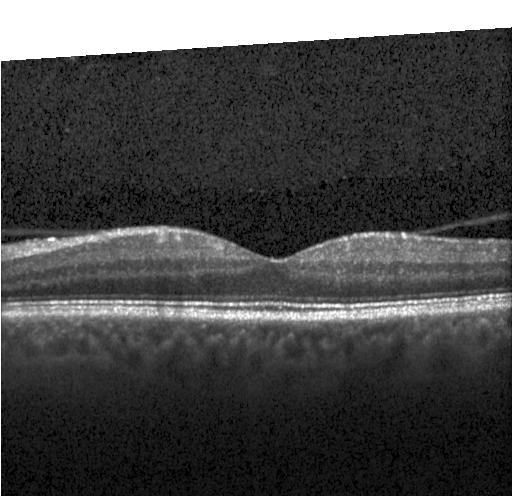

Diagnosis: no evidence of choroidal neovascularization, diabetic macular edema, or drusen.